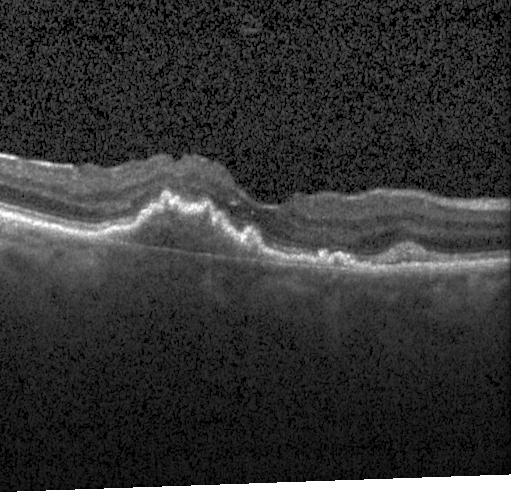
Spectral-domain OCT. OCT B-scan — Assessment: a choroidal neovascular membrane.